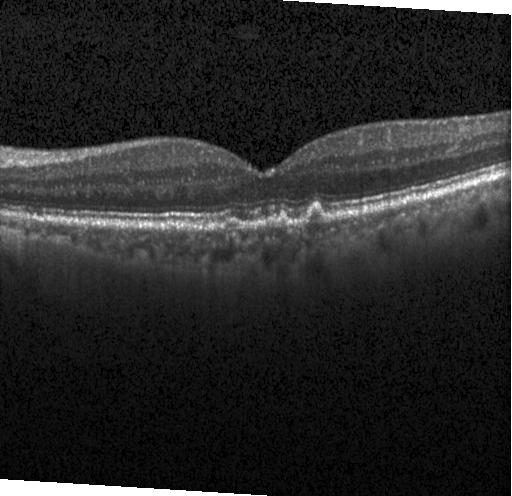 Acquired on a Heidelberg Spectralis. Optical coherence tomography B-scan — Diagnosis: multiple drusen.